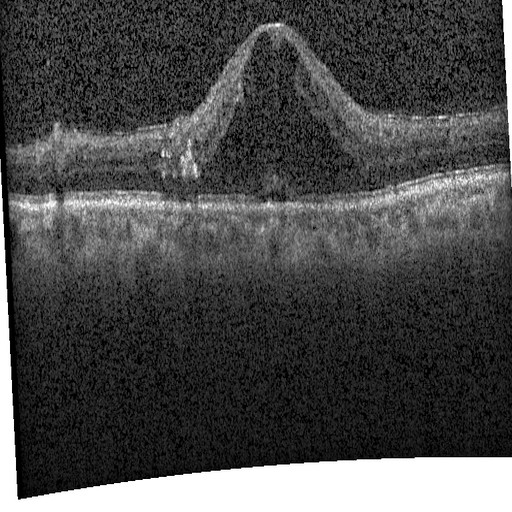

Optical coherence tomography B-scan · fovea-centered · Heidelberg Spectralis.
Diagnosis: diabetic macular edema (DME).